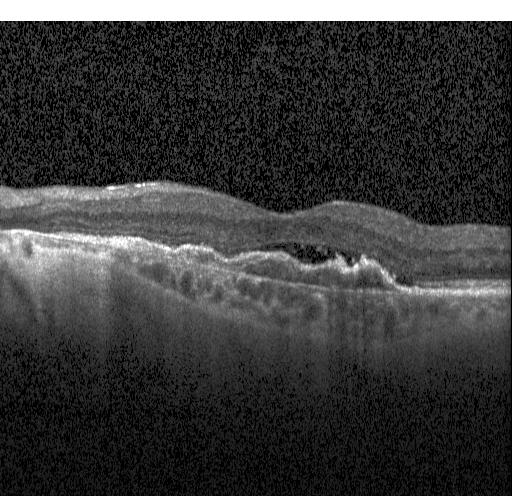 Choroidal neovascularization.